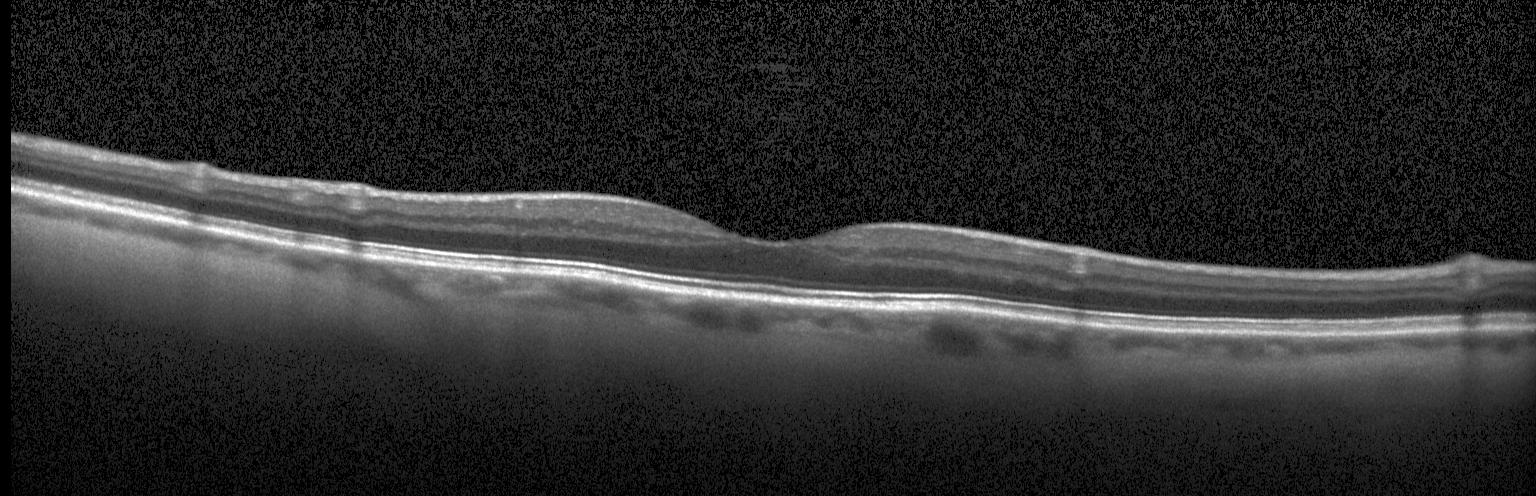 Optical coherence tomography B-scan; spectral-domain optical coherence tomography; fovea-centered; Heidelberg Spectralis
No choroidal neovascularization, no diabetic macular edema, and no drusen.